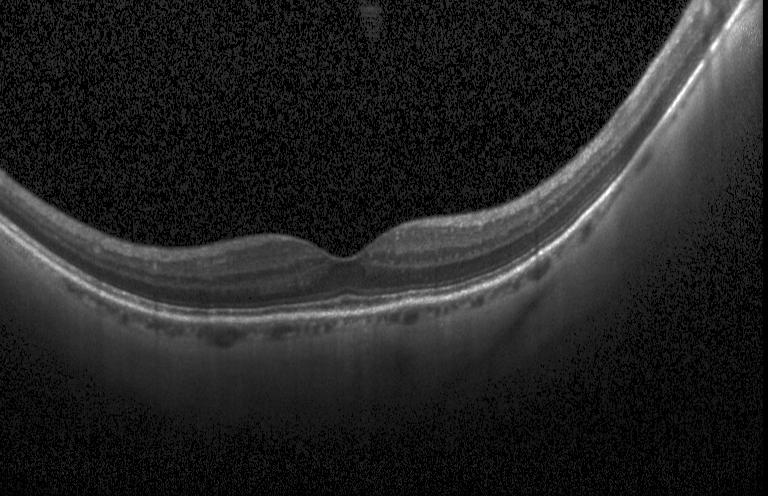

Finding: neither choroidal neovascularization, diabetic macular edema, nor drusen.